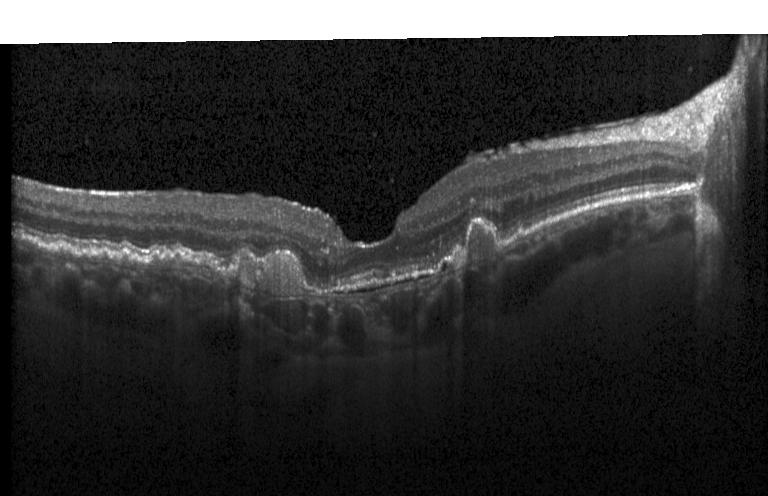 SD-OCT; fovea-centered; retinal OCT B-scan.
OCT finding: a choroidal neovascular membrane.